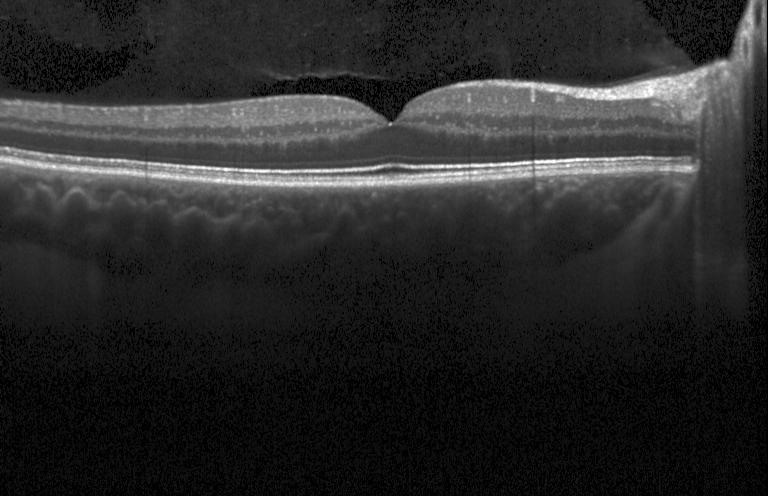

Optical coherence tomography scan; spectral-domain OCT; Heidelberg Spectralis OCT system; centered on the fovea. The scan shows neither choroidal neovascularization, diabetic macular edema, nor drusen.